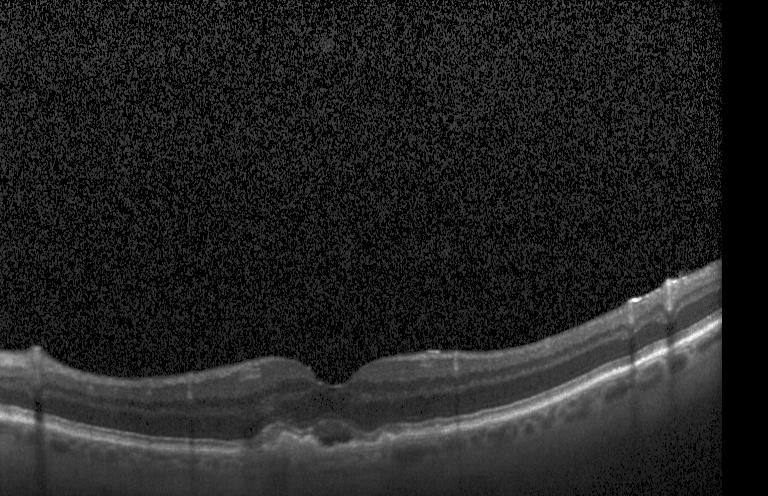
Dx: choroidal neovascularization.